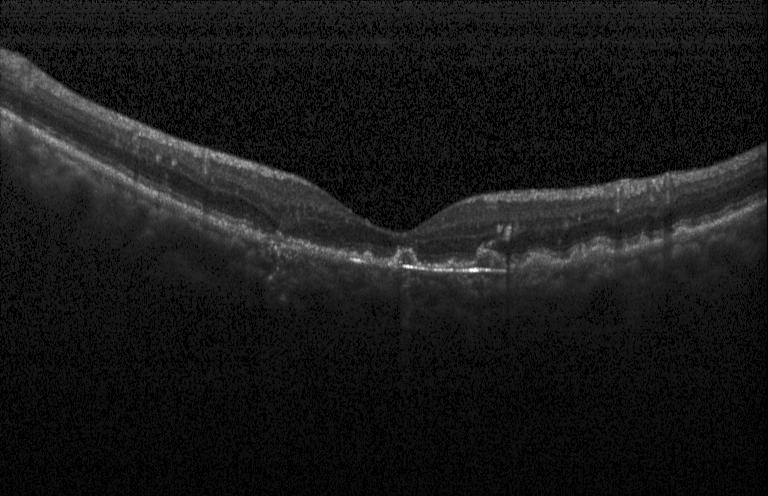
Spectral-domain optical coherence tomography. Heidelberg Spectralis OCT system. Optical coherence tomography B-scan. Centered on the fovea. This B-scan demonstrates a choroidal neovascular membrane.